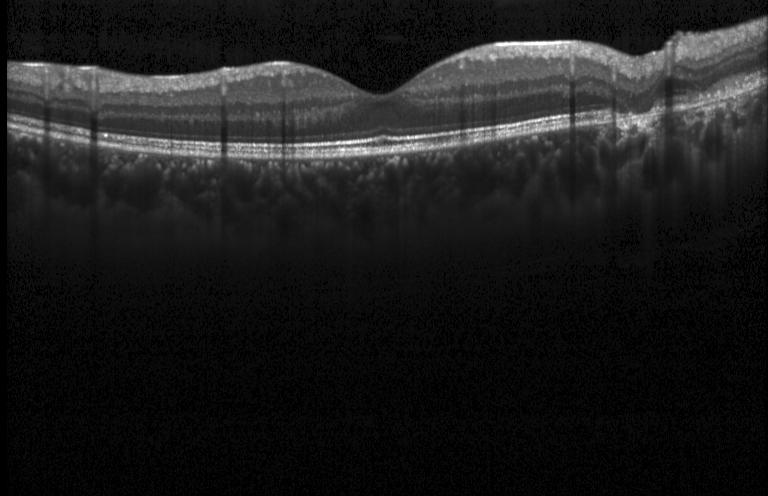
Retinal OCT cross-section showing no CNV, no DME, and no drusen.